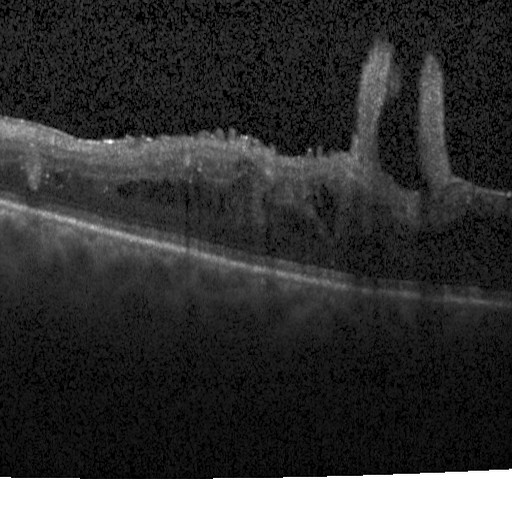
Retinal OCT B-scan — Macular OCT: diabetic macular edema.